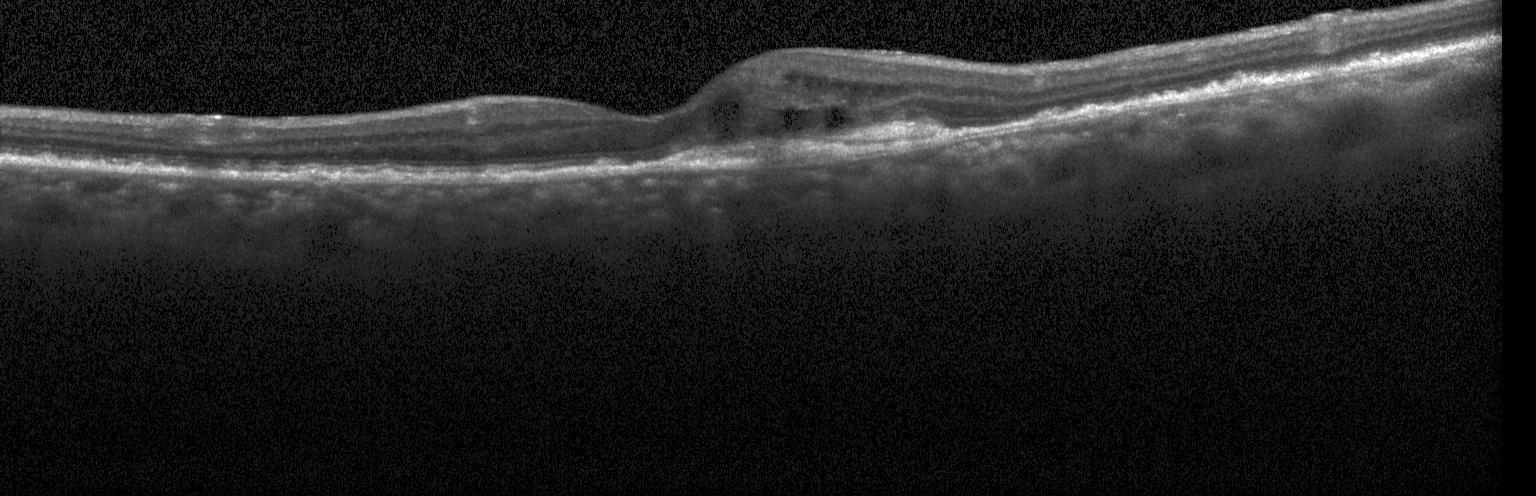

Diagnosis: CNV.